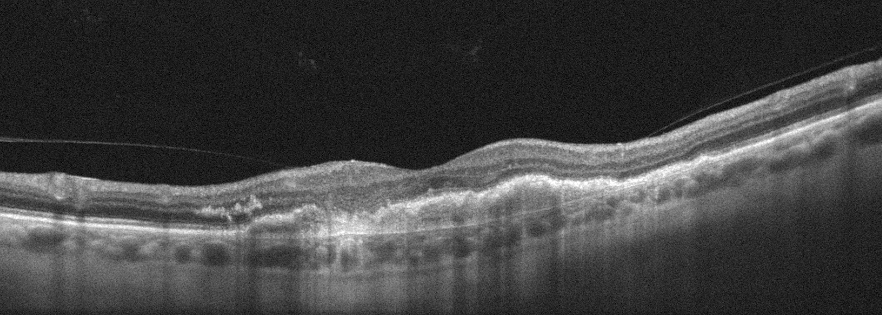
Retinal OCT B-scan, OD, instrument: Optovue Avanti RTVue XR, macular scan. This B-scan demonstrates AMD.